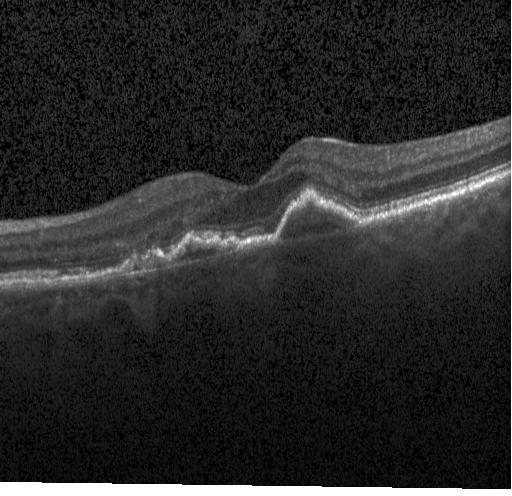
Dx: choroidal neovascularization.